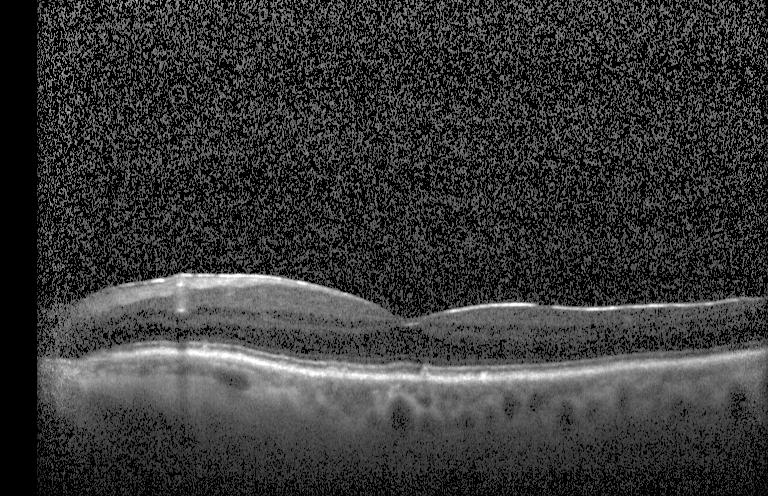
Diagnosis: sub-RPE drusenoid deposits.